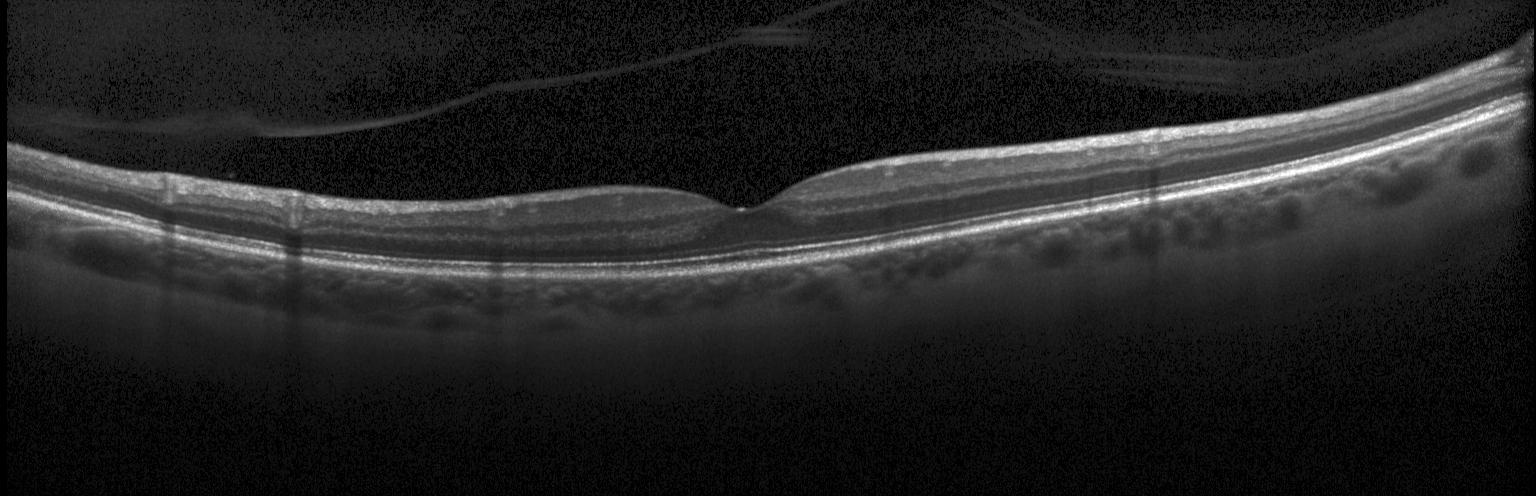 OCT line scan. Macular OCT: no choroidal neovascularization, no diabetic macular edema, and no drusen.